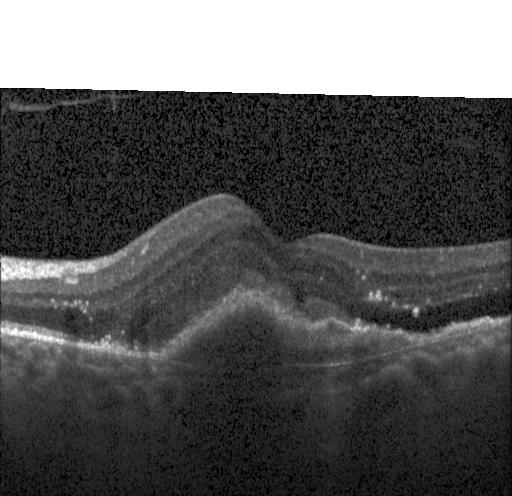
Optical coherence tomography scan · SD-OCT.
Assessment: a choroidal neovascular membrane.